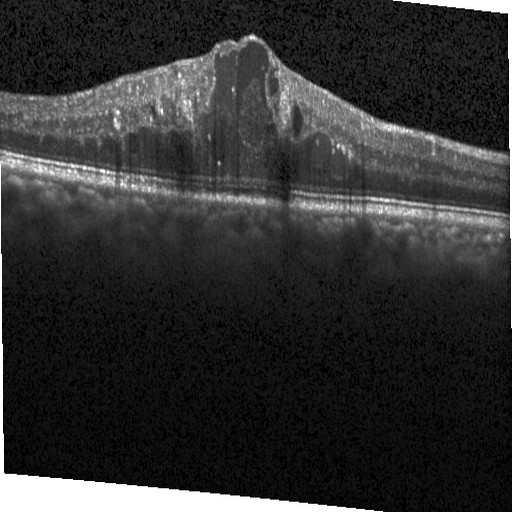 SD-OCT; macular scan; retinal OCT cross-section; instrument: Heidelberg Spectralis
Finding: diabetic macular edema (DME).